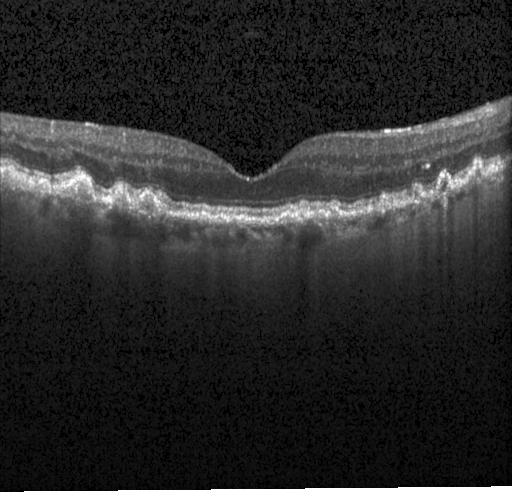

Heidelberg Spectralis OCT system. Fovea-centered. SD-OCT. Retinal OCT cross-section — OCT finding: drusen.